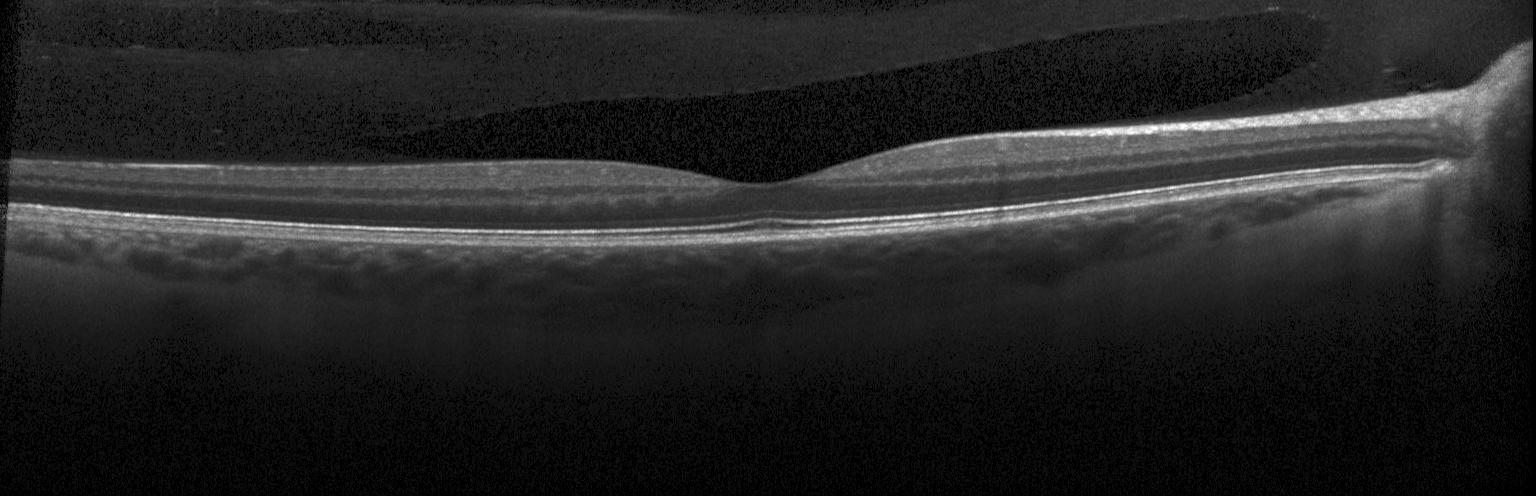 Spectral-domain optical coherence tomography; optical coherence tomography scan; macular scan; Heidelberg Spectralis
Neither choroidal neovascularization, diabetic macular edema, nor drusen.